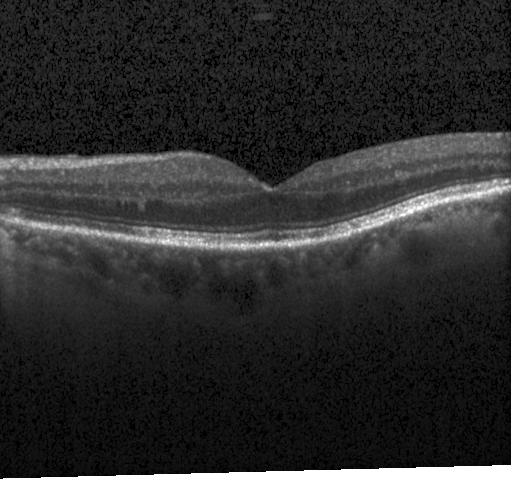
Heidelberg Spectralis OCT system. Retinal OCT cross-section. Centered on the fovea. Impression: no choroidal neovascularization, diabetic macular edema, or drusen.